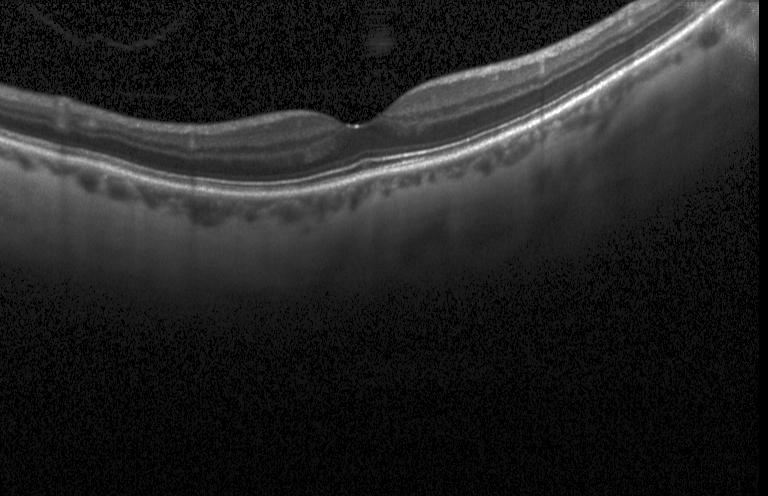

Finding: no choroidal neovascularization, no diabetic macular edema, and no drusen.